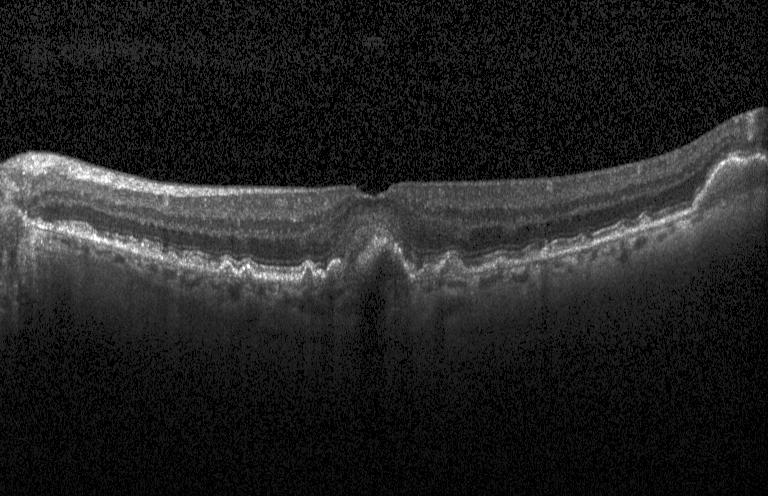

Optical coherence tomography B-scan.
OCT finding: a choroidal neovascular membrane.